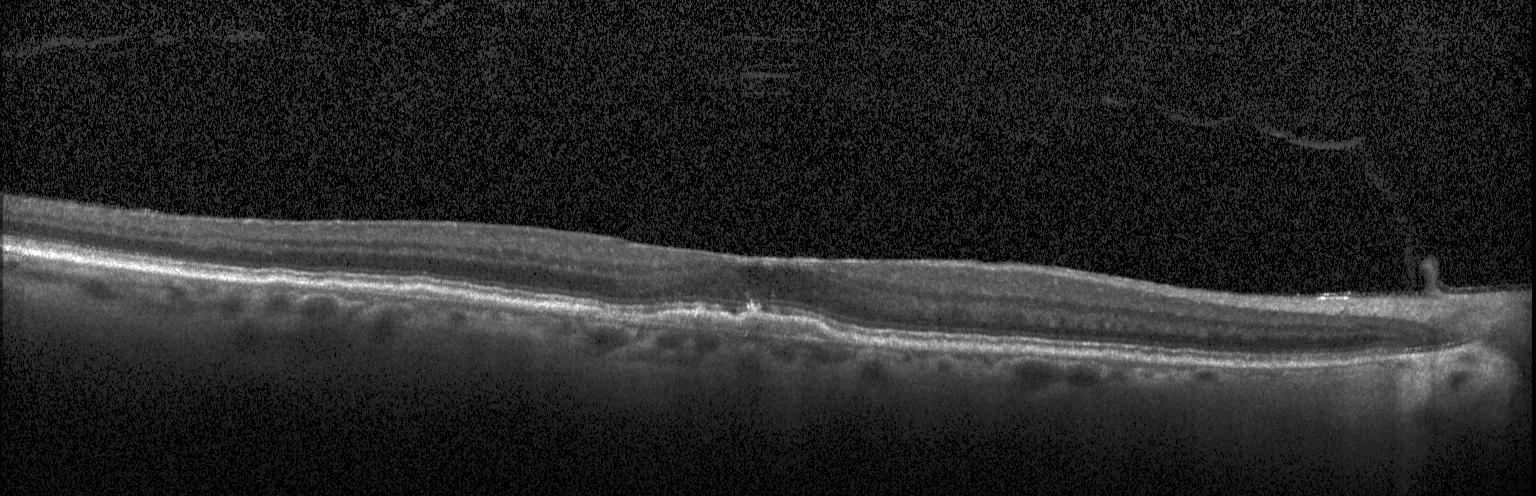
Spectral-domain OCT B-scan: choroidal neovascularization (CNV).